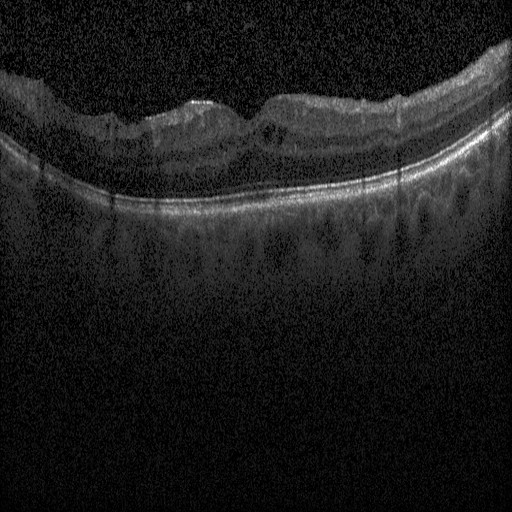
Retinal OCT cross-section
OCT finding: diabetic macular edema.